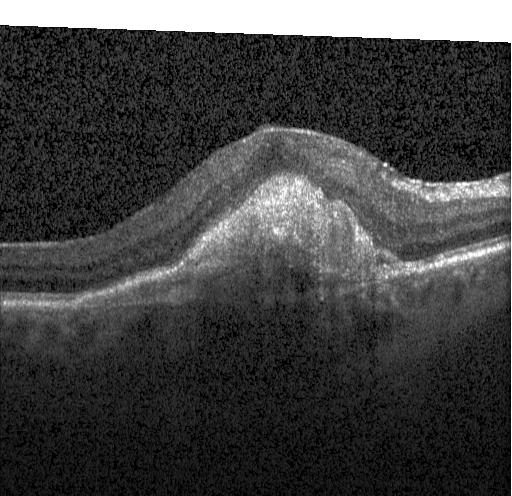 Spectral-domain OCT B-scan: a choroidal neovascular membrane.